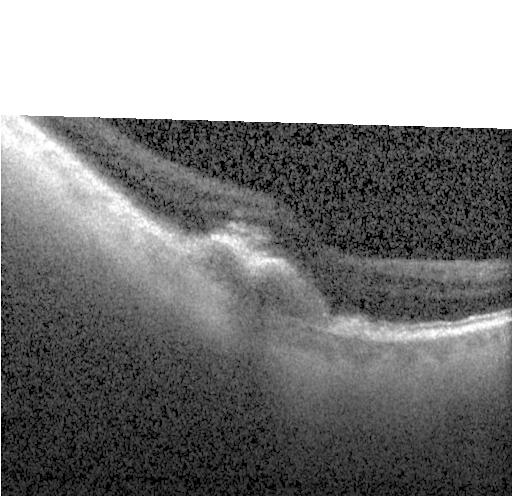
Macular OCT demonstrating CNV.